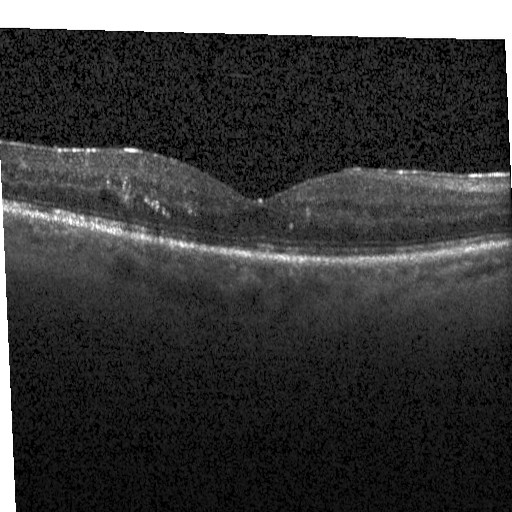
This B-scan demonstrates DME.